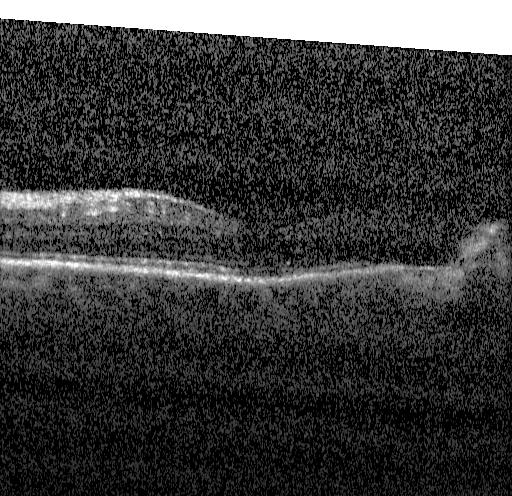

Macular scan; optical coherence tomography B-scan — Diagnosis: a choroidal neovascular membrane.